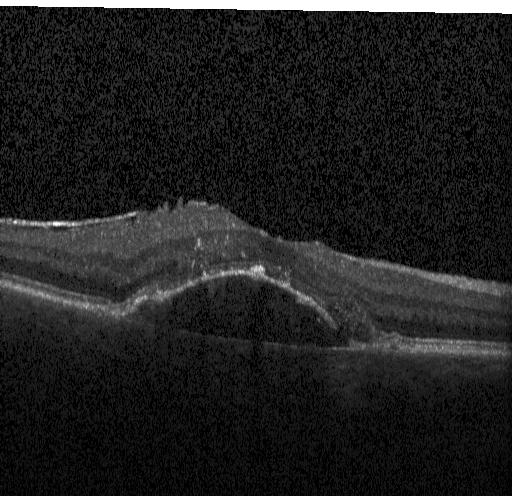

Retinal OCT B-scan · spectral-domain optical coherence tomography. Dx: choroidal neovascularization (CNV).